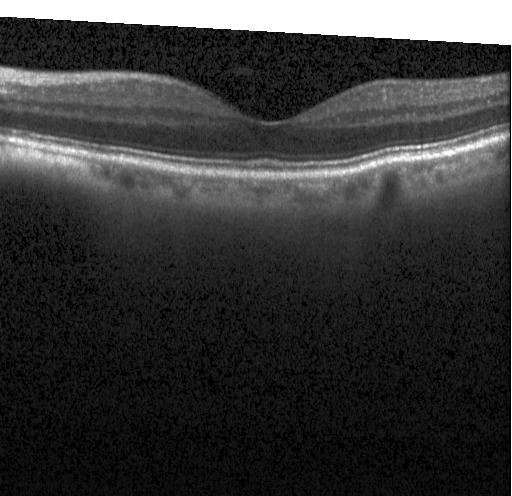
Dx: no choroidal neovascularization, diabetic macular edema, or drusen.